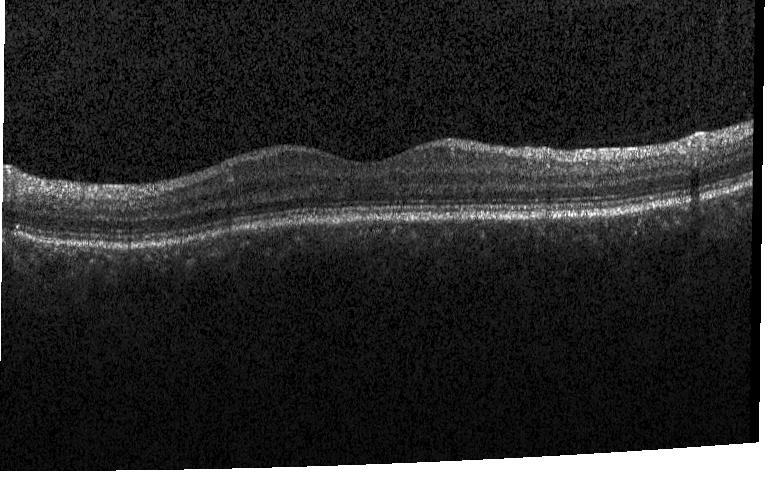
Diagnosis: no choroidal neovascularization, no diabetic macular edema, and no drusen.